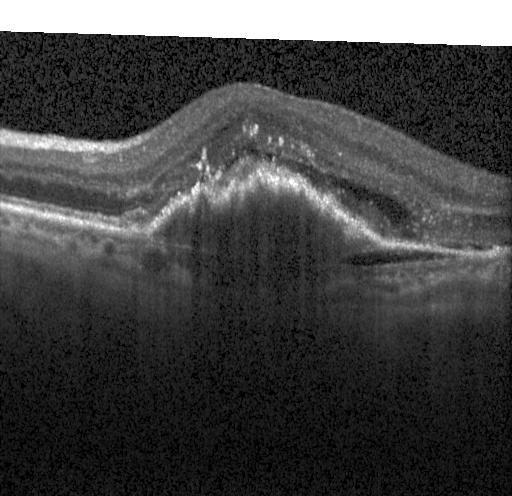 Spectral-domain OCT. Horizontal scan through the fovea. OCT line scan. Heidelberg Spectralis — Diagnosis: CNV.